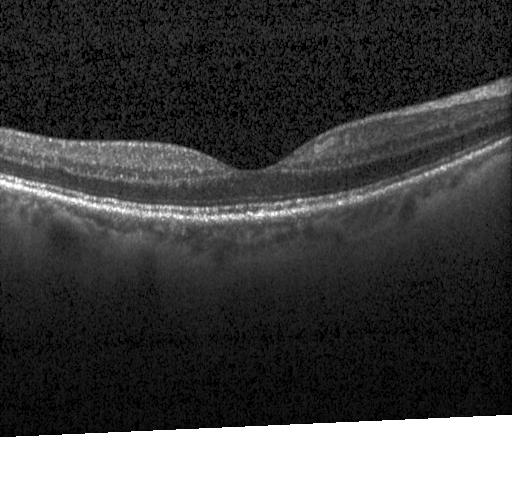
OCT finding: no choroidal neovascularization, no diabetic macular edema, and no drusen.